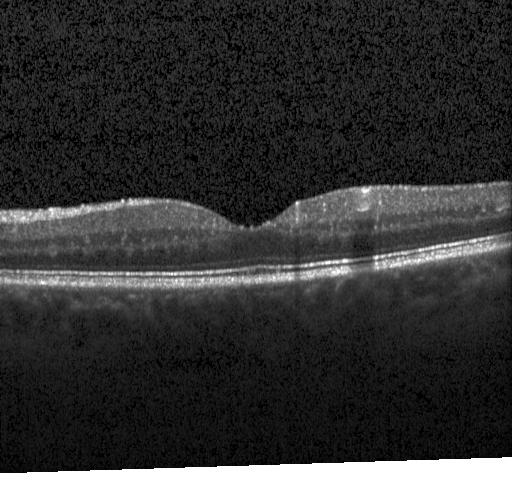

Diagnosis: no CNV, DME, or drusen.